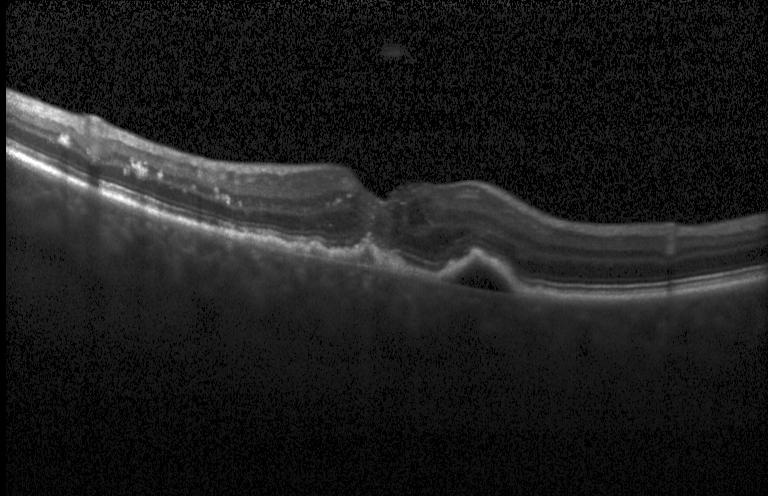

Acquired on a Heidelberg Spectralis · OCT B-scan.
This B-scan demonstrates a choroidal neovascular membrane.